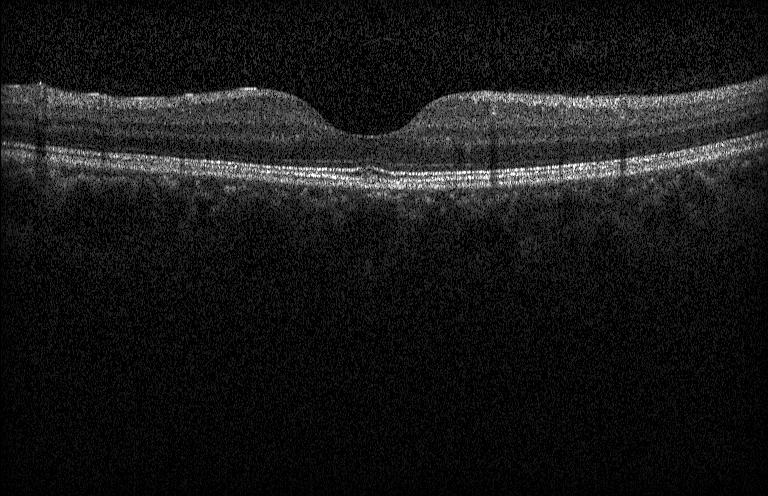 Through the macula, SD-OCT, optical coherence tomography scan.
This B-scan demonstrates no choroidal neovascularization, diabetic macular edema, or drusen.